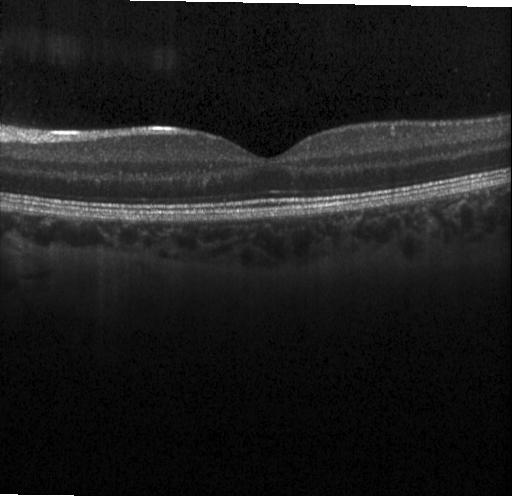 Retinal OCT cross-section, Heidelberg Spectralis OCT system
Assessment: no choroidal neovascularization, no diabetic macular edema, and no drusen.